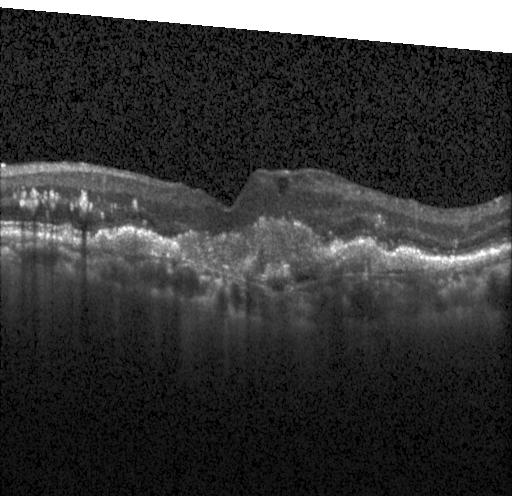
Assessment: choroidal neovascularization (CNV).